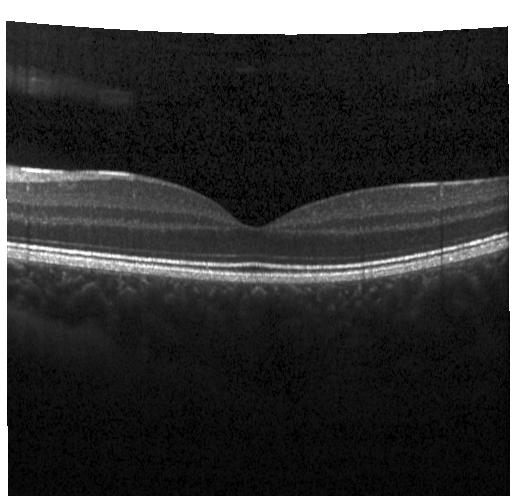 No CNV, no DME, and no drusen.